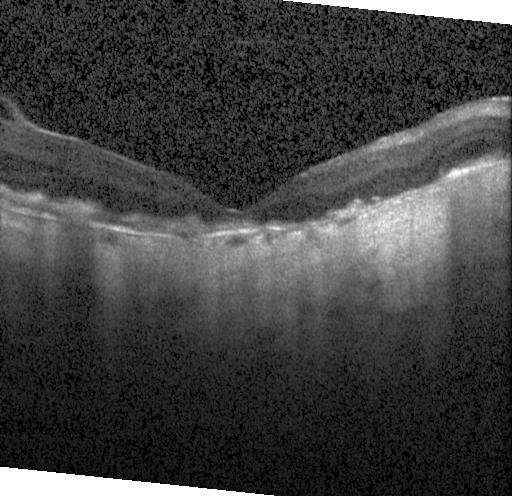

Spectral-domain OCT B-scan: a choroidal neovascular membrane.